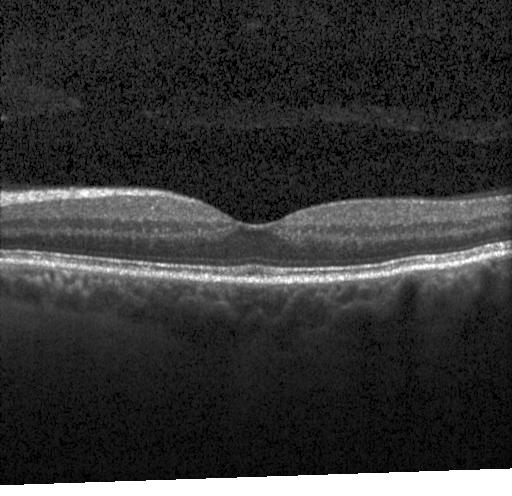 Optical coherence tomography B-scan — Finding: no choroidal neovascularization, no diabetic macular edema, and no drusen.